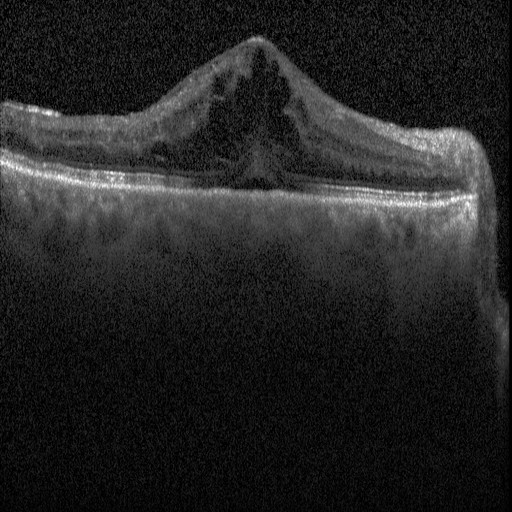

OCT line scan. Finding: DME.